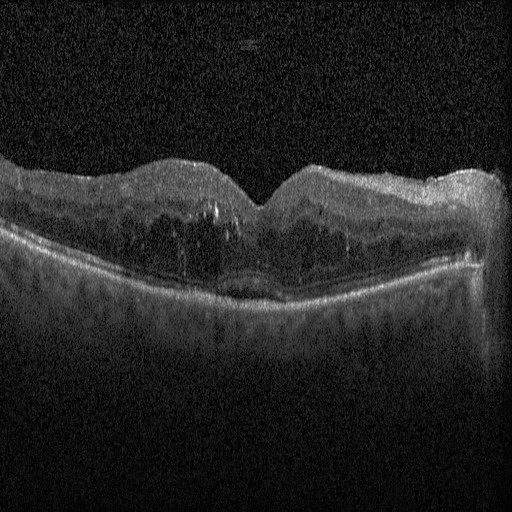
Spectral-domain OCT; acquired on a Heidelberg Spectralis; fovea-centered; retinal OCT cross-section
DME.